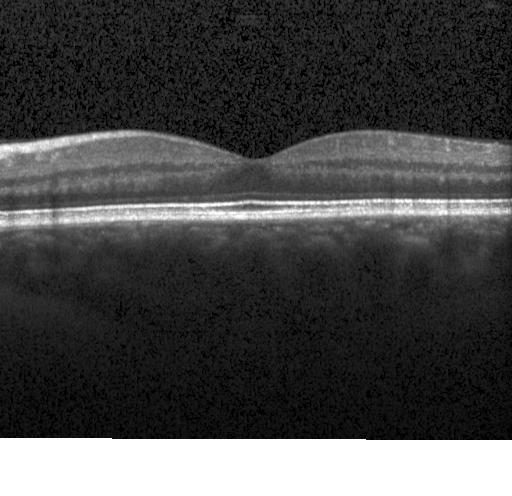

Dx: no choroidal neovascularization, no diabetic macular edema, and no drusen.